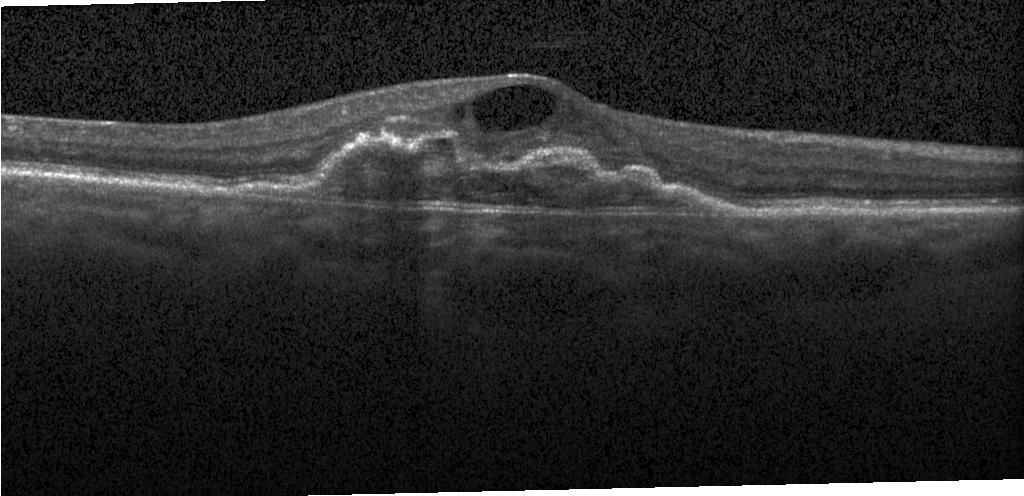 Retinal OCT cross-section showing CNV.